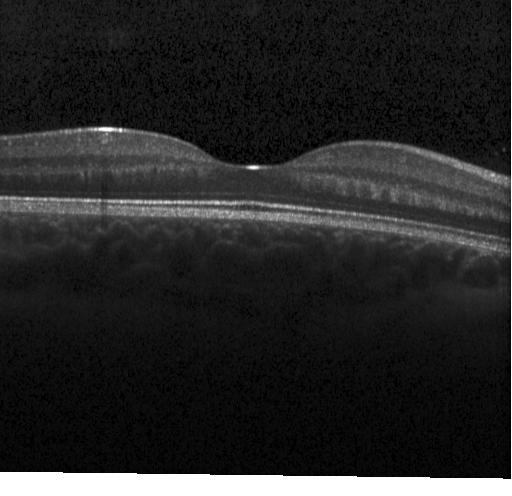

Neither choroidal neovascularization, diabetic macular edema, nor drusen.